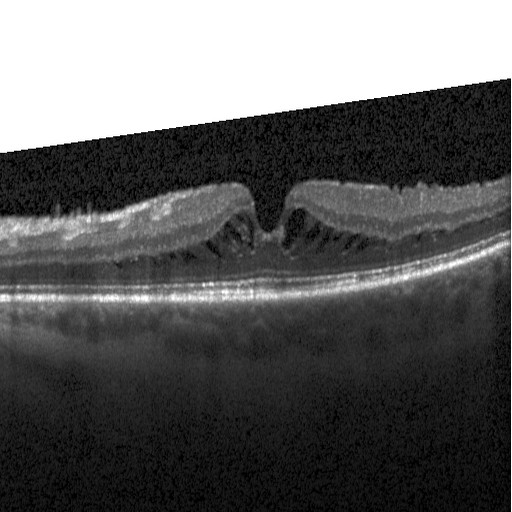
Heidelberg Spectralis OCT system; retinal OCT cross-section; spectral-domain OCT; fovea-centered. Macular OCT: diabetic macular edema (DME).